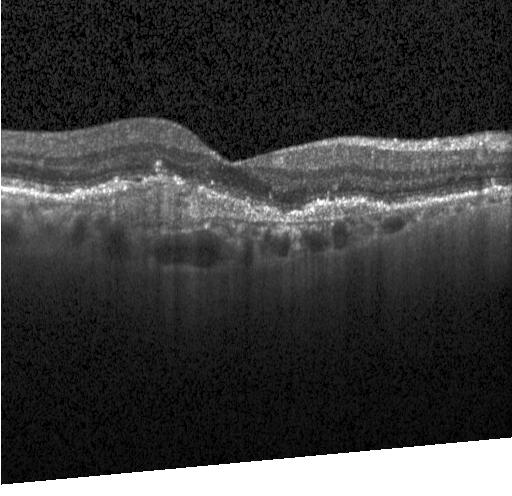
Spectral-domain OCT · optical coherence tomography scan · horizontal scan through the fovea · acquired on a Heidelberg Spectralis — Finding: a choroidal neovascular membrane.